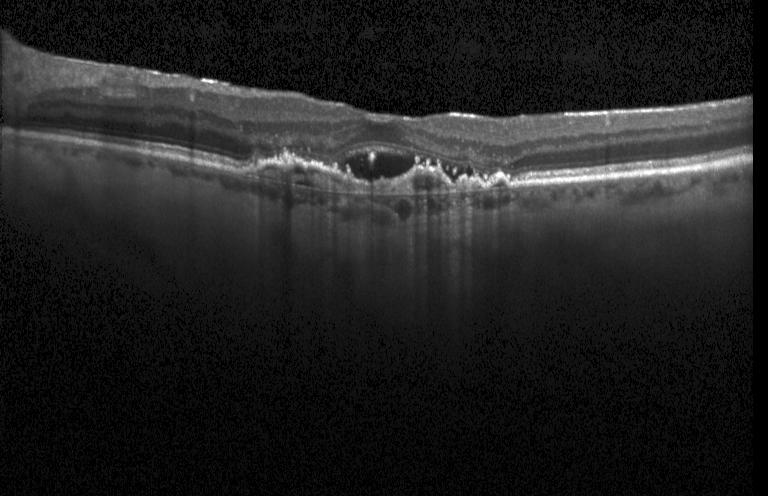

Retinal OCT cross-section. Instrument: Heidelberg Spectralis — OCT finding: choroidal neovascularization.